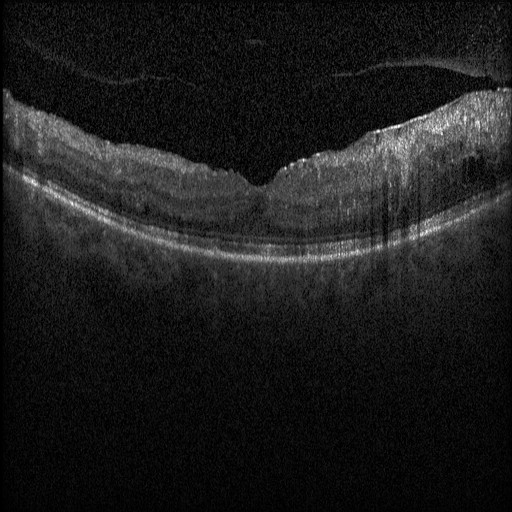

Diagnosis: diabetic macular edema.